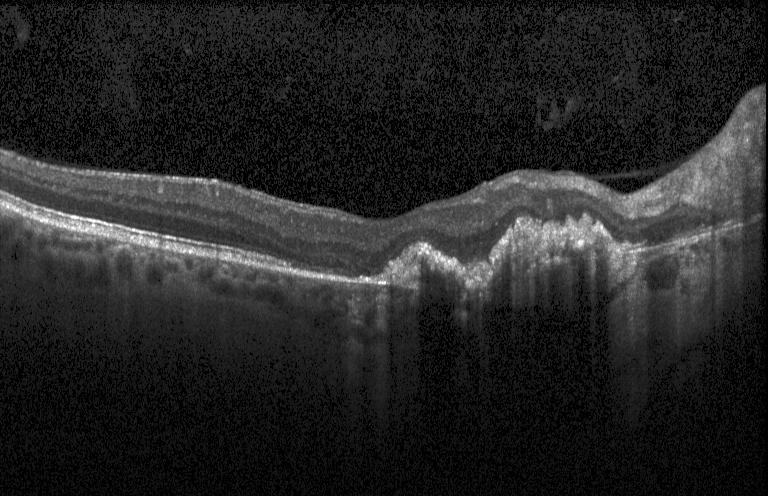

Optical coherence tomography B-scan.
Impression: choroidal neovascularization (CNV).